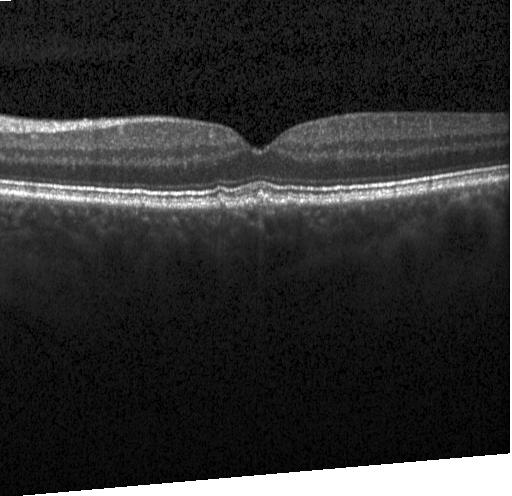

Optical coherence tomography B-scan — Assessment: sub-RPE drusenoid deposits.